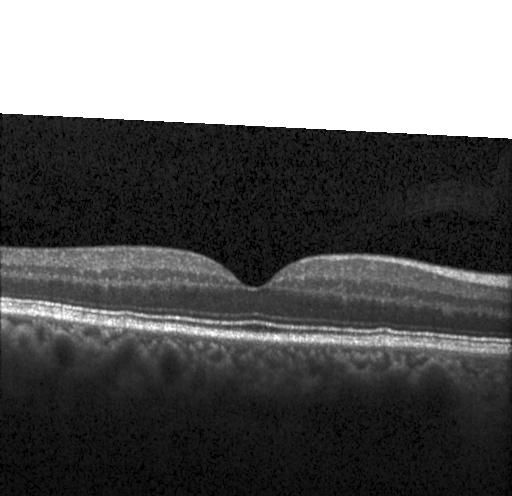 OCT line scan
Impression: no choroidal neovascularization, no diabetic macular edema, and no drusen.